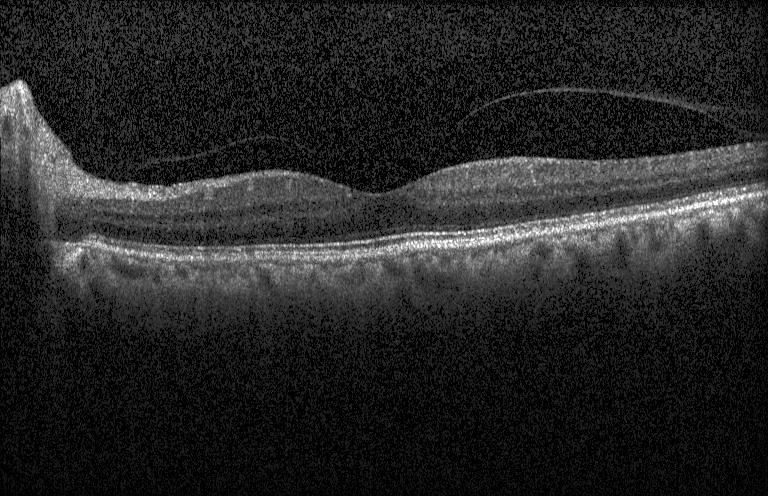
Optical coherence tomography B-scan.
Macular OCT: neither choroidal neovascularization, diabetic macular edema, nor drusen.